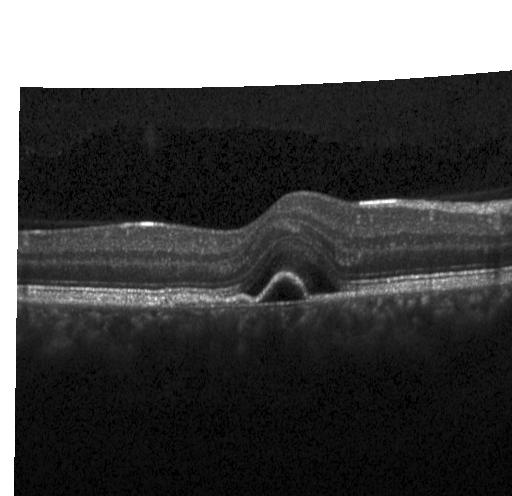

OCT line scan.
Dx: choroidal neovascularization.